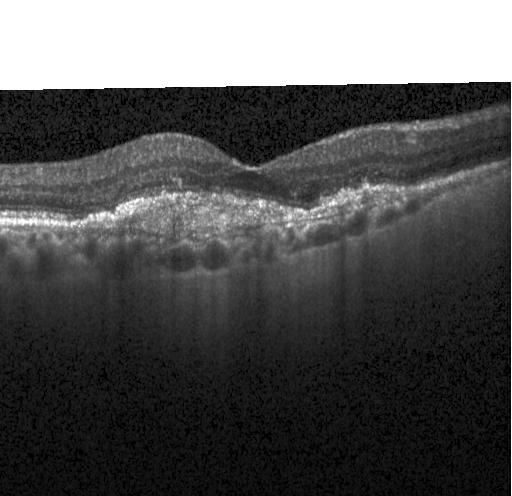 Dx: choroidal neovascularization (CNV).